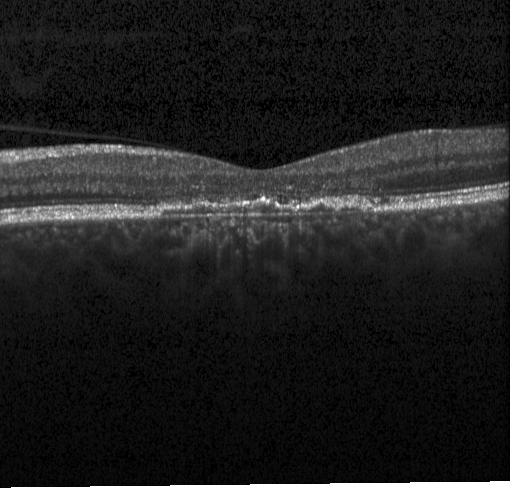 OCT B-scan showing a choroidal neovascular membrane.